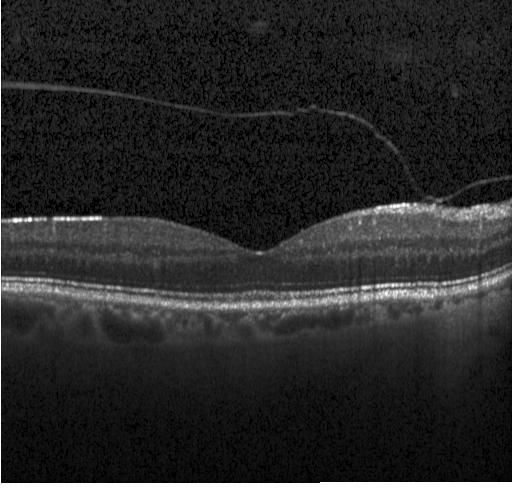
Finding: no evidence of choroidal neovascularization, diabetic macular edema, or drusen.